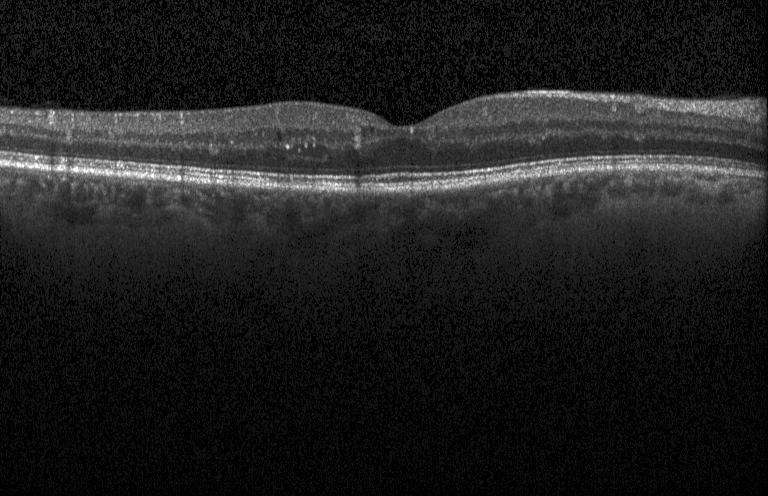

OCT B-scan. Heidelberg Spectralis OCT system. Spectral-domain OCT.
Assessment: neither CNV, DME, nor drusen.